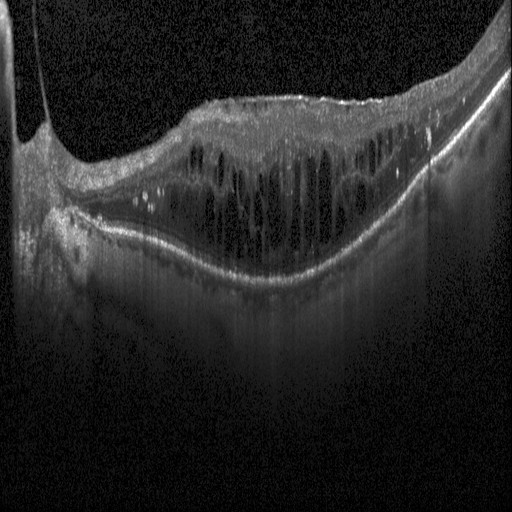
Fovea-centered, optical coherence tomography scan
Diabetic macular edema (DME).